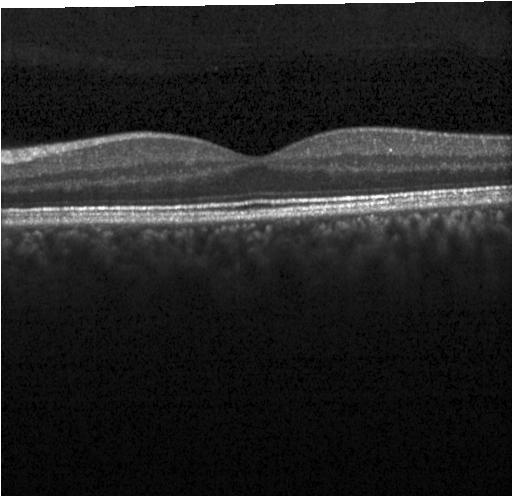
Finding: no CNV, no DME, and no drusen.